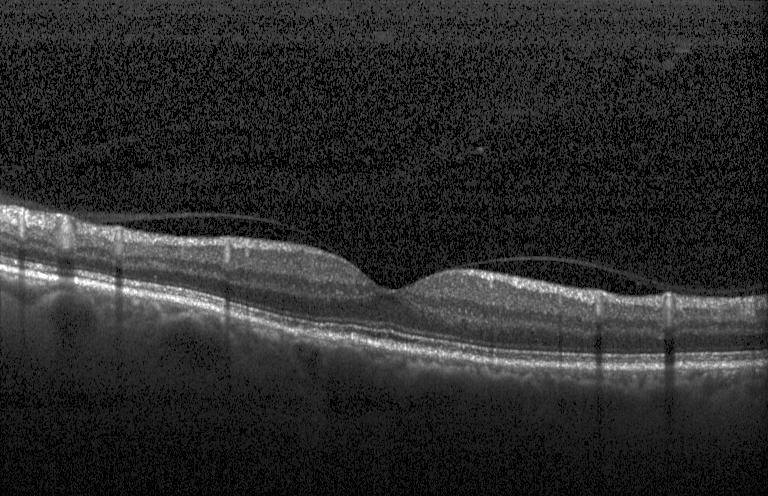 Heidelberg Spectralis OCT system. OCT B-scan. Horizontal scan through the fovea. SD-OCT — Impression: neither choroidal neovascularization, diabetic macular edema, nor drusen.